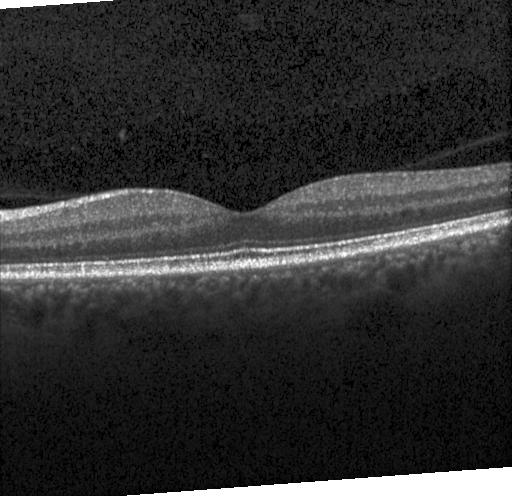
Finding: no evidence of choroidal neovascularization, diabetic macular edema, or drusen.